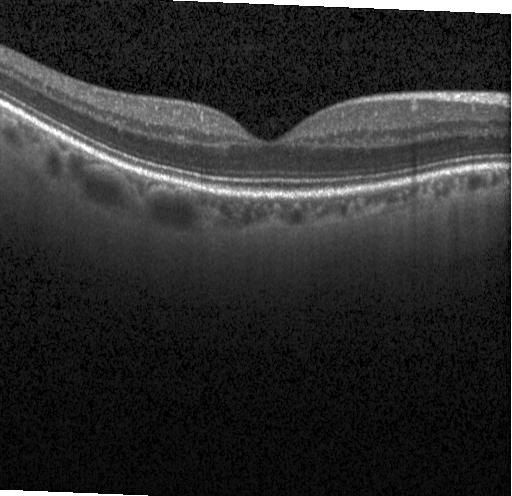 Optical coherence tomography scan. SD-OCT
Finding: no choroidal neovascularization, no diabetic macular edema, and no drusen.